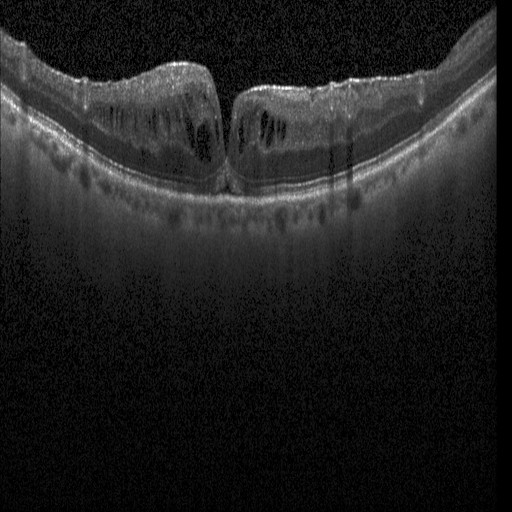 Heidelberg Spectralis; retinal OCT cross-section. Finding: DME.